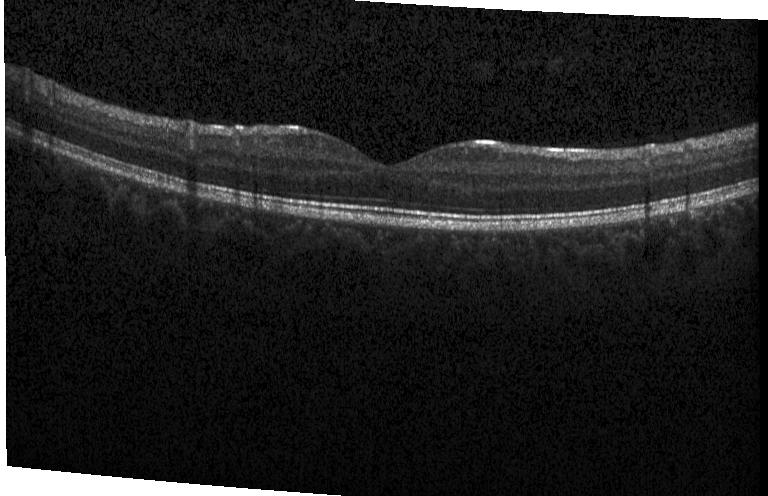
Dx: no evidence of CNV, DME, or drusen.